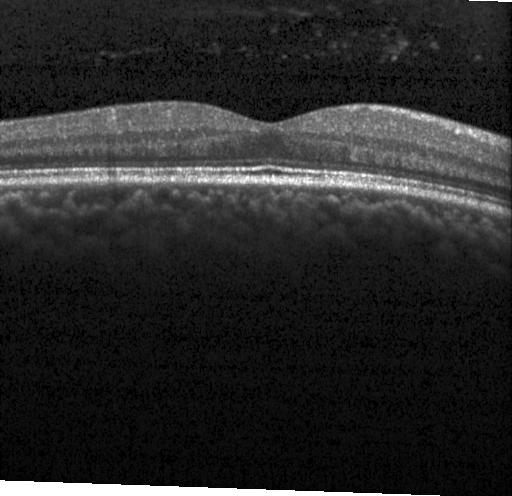
Optical coherence tomography B-scan
This B-scan demonstrates no choroidal neovascularization, no diabetic macular edema, and no drusen.